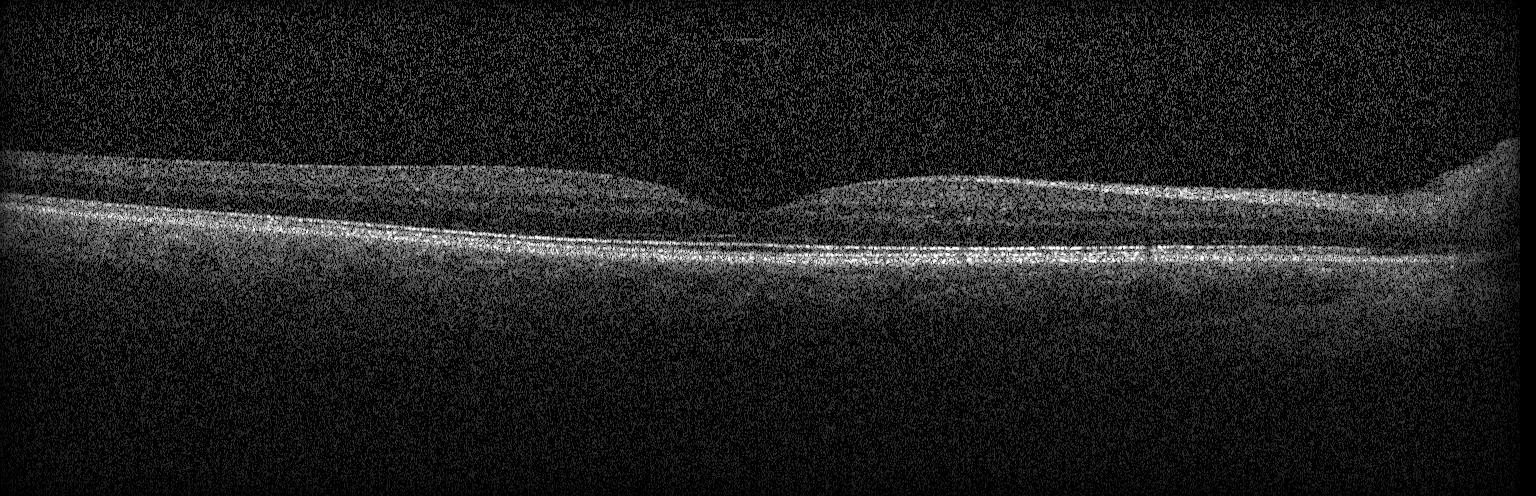
Diagnosis: neither choroidal neovascularization, diabetic macular edema, nor drusen.